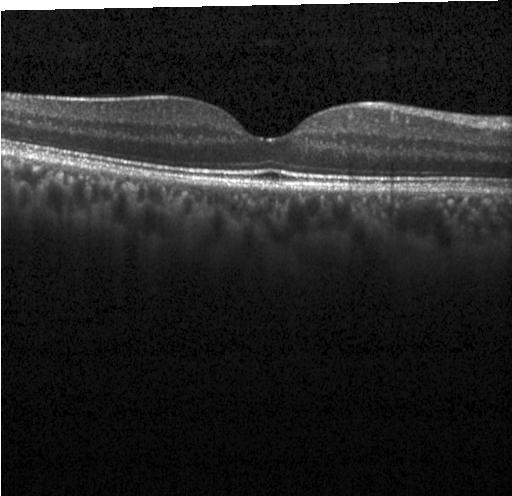 The scan shows neither choroidal neovascularization, diabetic macular edema, nor drusen.